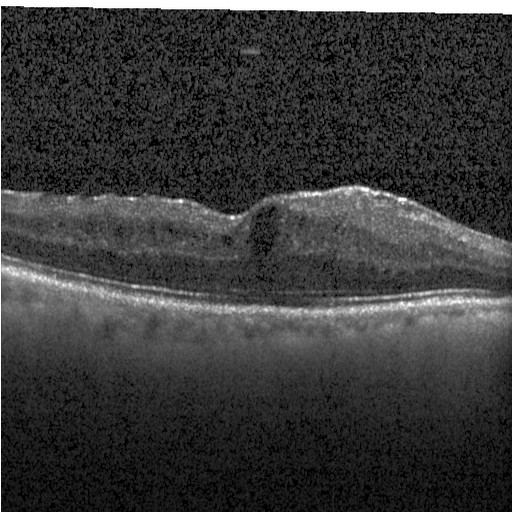
SD-OCT; through the macula; retinal OCT B-scan; Heidelberg Spectralis OCT system. Assessment: DME.